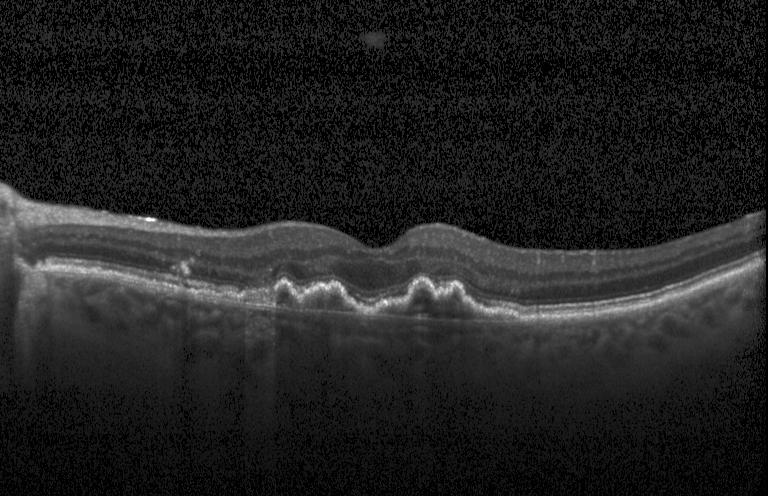
Retinal OCT B-scan. SD-OCT. Centered on the fovea.
Impression: choroidal neovascularization.